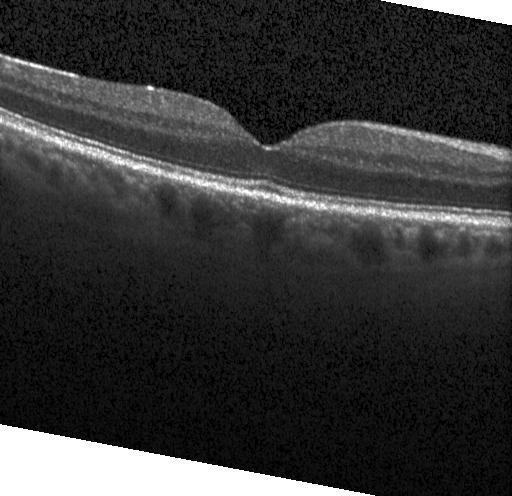
Optical coherence tomography B-scan. The scan shows no choroidal neovascularization, no diabetic macular edema, and no drusen.